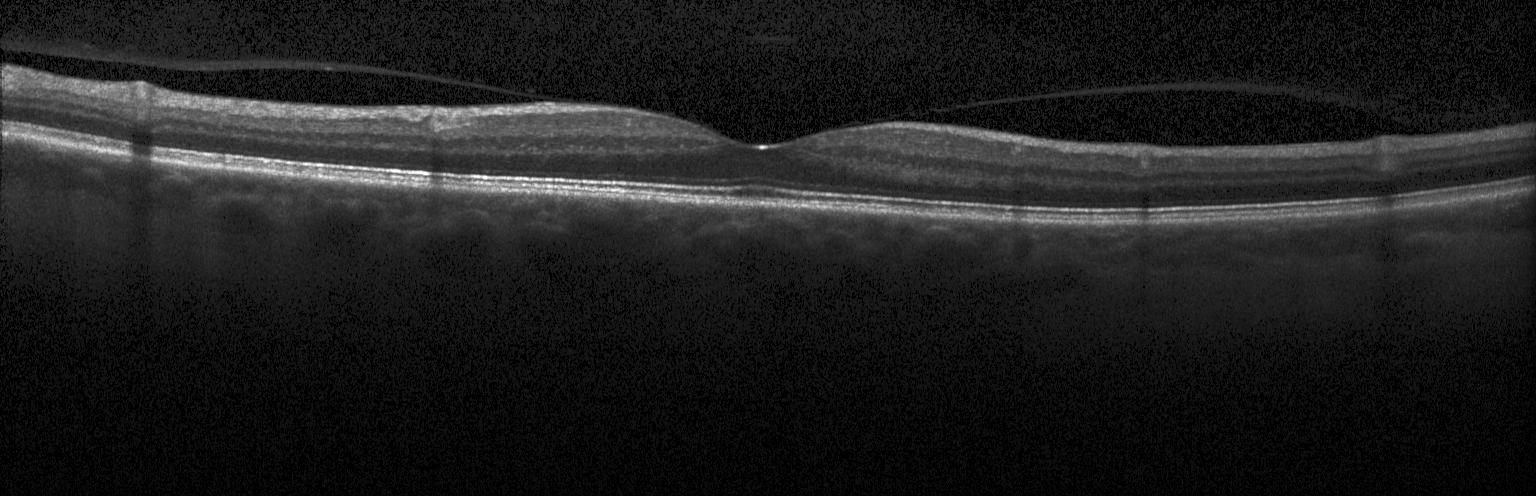

Spectral-domain OCT · acquired on a Heidelberg Spectralis · optical coherence tomography scan · macular scan
Finding: neither CNV, DME, nor drusen.